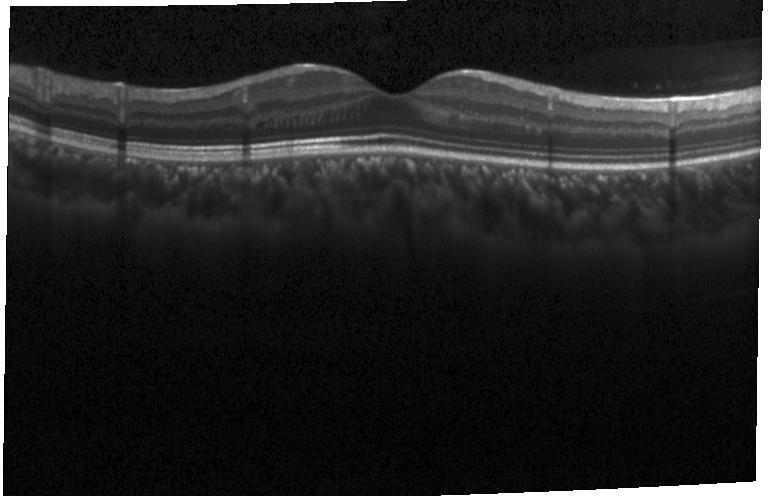

Finding: no choroidal neovascularization, diabetic macular edema, or drusen.